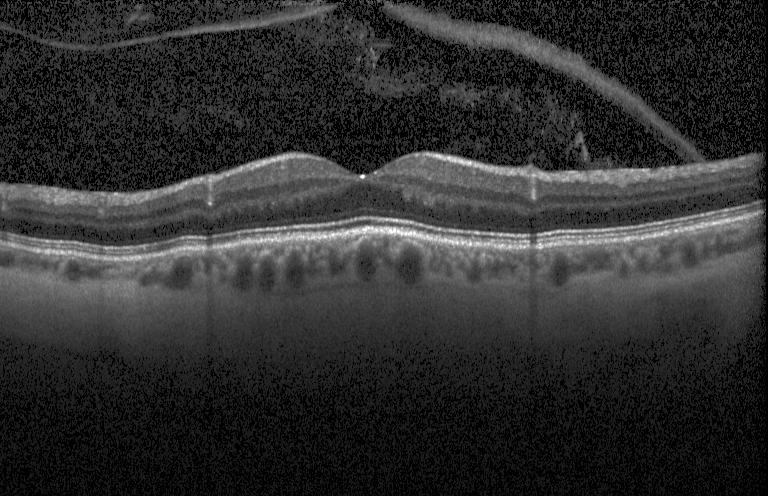 Retinal OCT cross-section, Heidelberg Spectralis, spectral-domain OCT
No evidence of choroidal neovascularization, diabetic macular edema, or drusen.